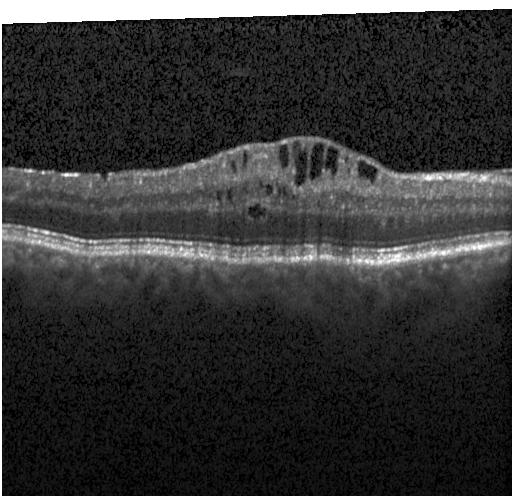
The scan shows DME.